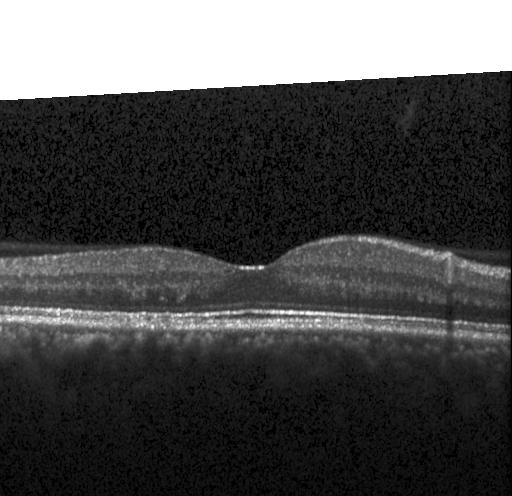

Horizontal scan through the fovea; OCT line scan.
Finding: no evidence of choroidal neovascularization, diabetic macular edema, or drusen.